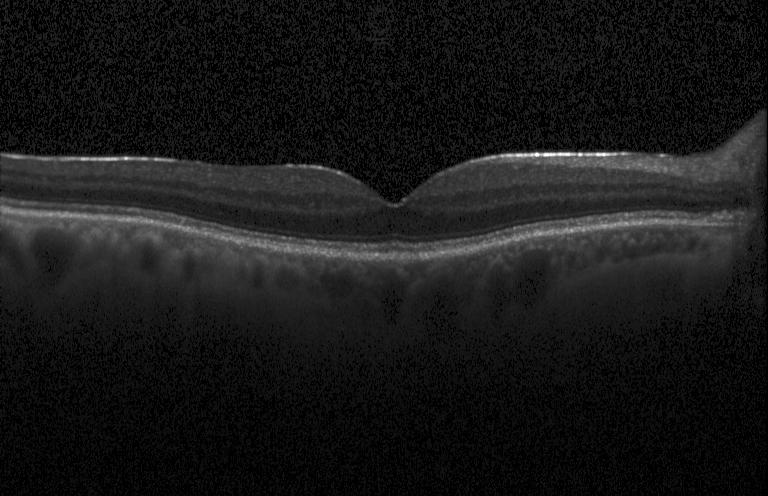 Instrument: Heidelberg Spectralis · retinal OCT cross-section.
This B-scan demonstrates no choroidal neovascularization, no diabetic macular edema, and no drusen.